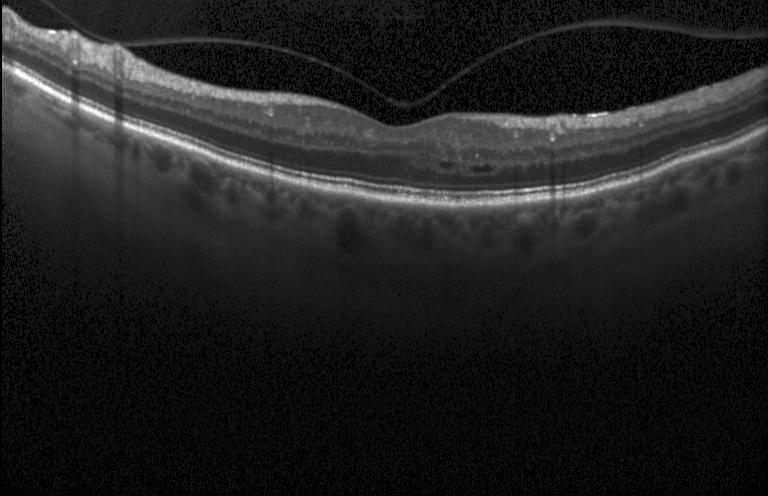
Retinal OCT cross-section; spectral-domain optical coherence tomography — OCT finding: DME.